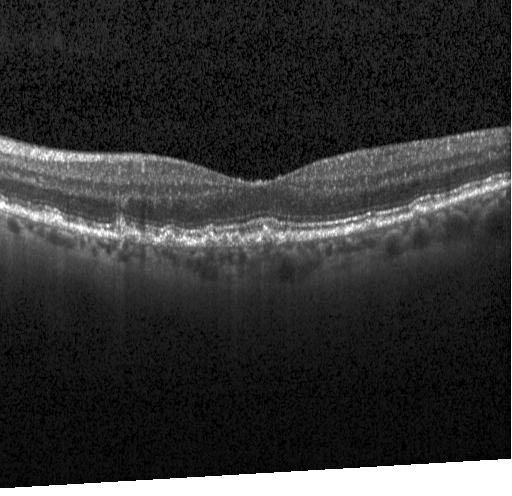

Diagnosis: drusen.